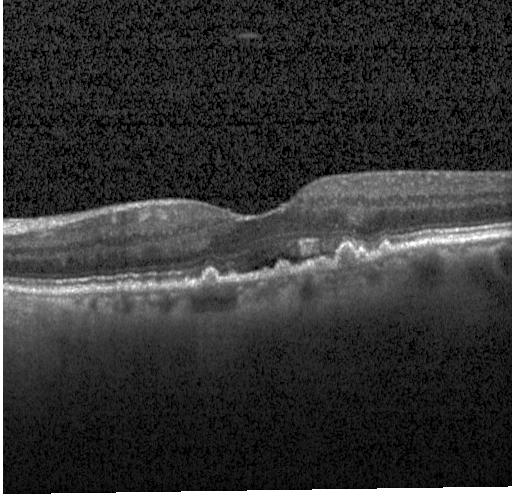

Impression: a choroidal neovascular membrane.